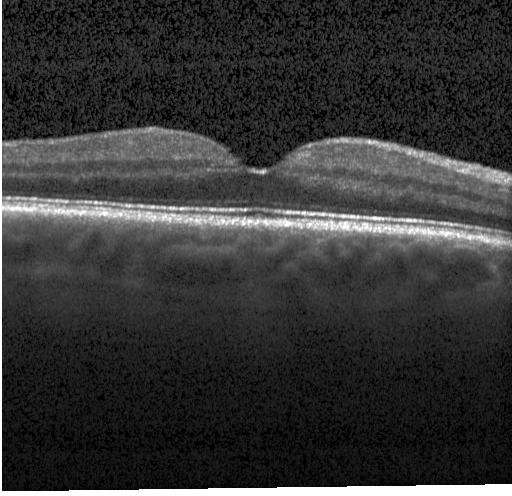 SD-OCT, retinal OCT B-scan, Heidelberg Spectralis OCT system, centered on the fovea.
Neither choroidal neovascularization, diabetic macular edema, nor drusen.